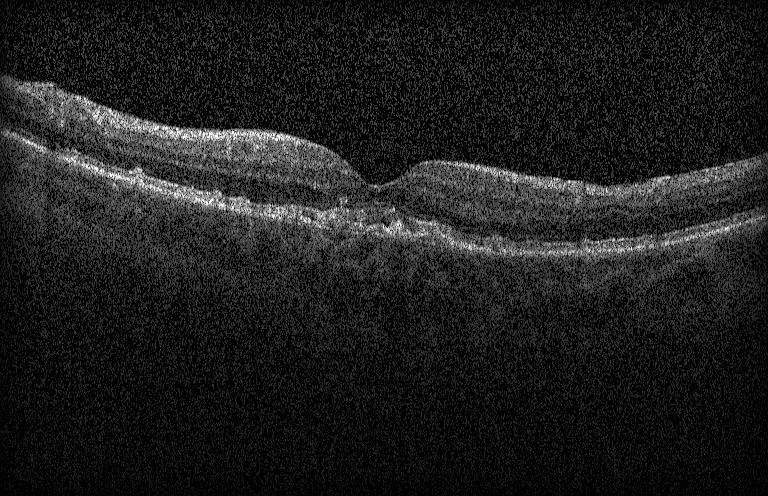 Retinal OCT cross-section. Macular scan. Spectral-domain optical coherence tomography.
This B-scan demonstrates choroidal neovascularization (CNV).